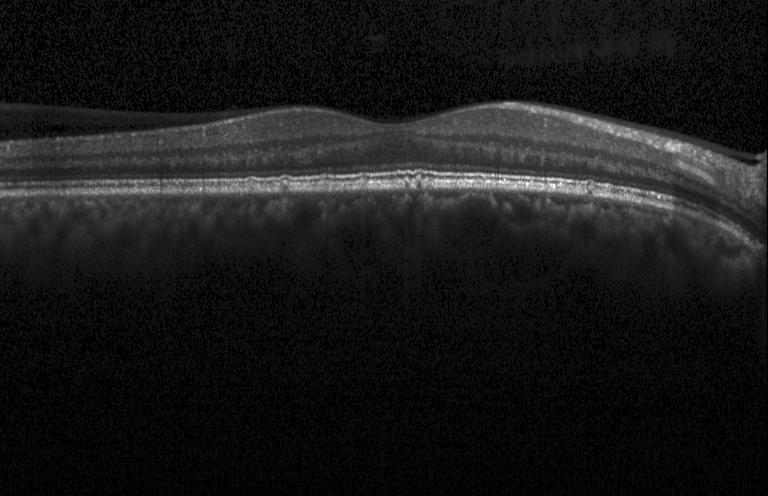 Macular OCT: drusen.